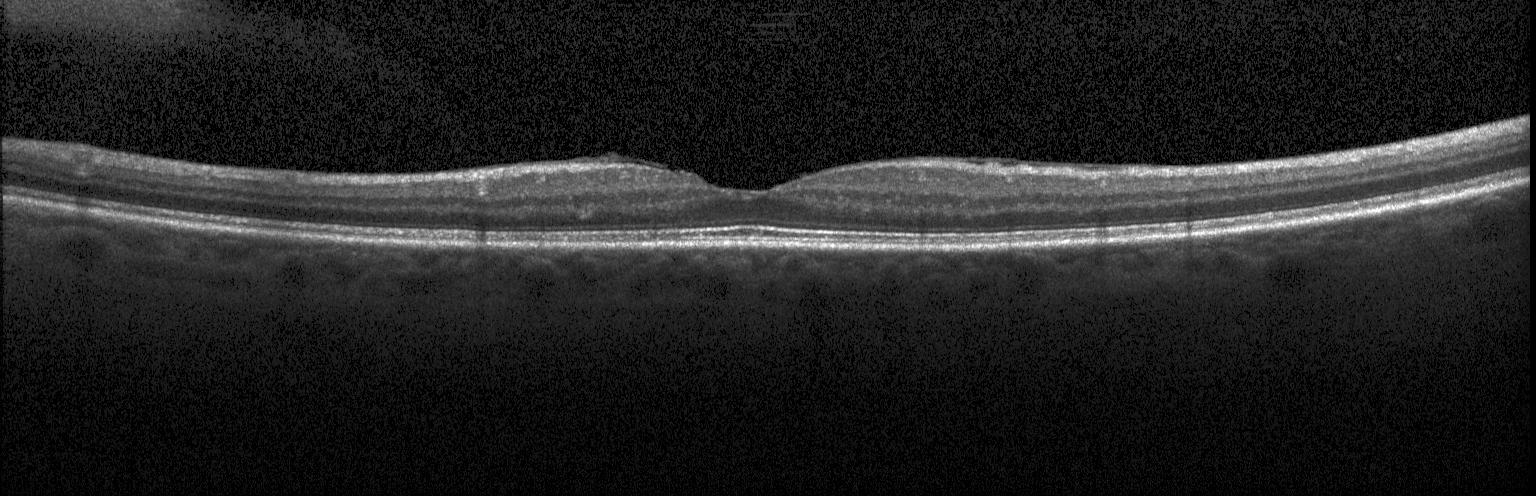
Optical coherence tomography B-scan. This B-scan demonstrates no evidence of choroidal neovascularization, diabetic macular edema, or drusen.